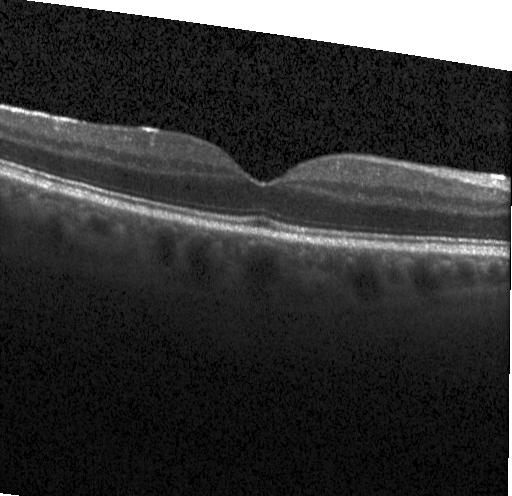

Optical coherence tomography B-scan · spectral-domain OCT — Impression: no CNV, no DME, and no drusen.